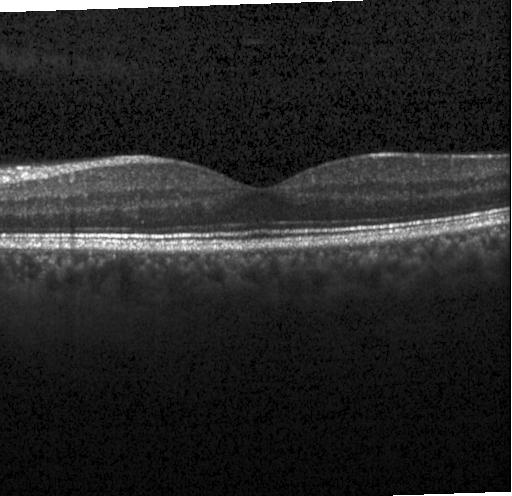
This B-scan demonstrates neither CNV, DME, nor drusen.